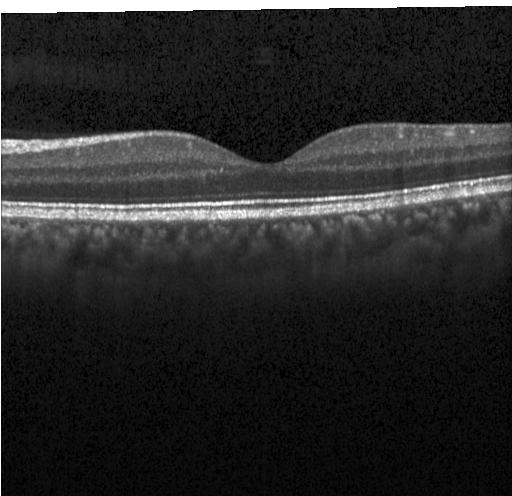

The scan shows no evidence of choroidal neovascularization, diabetic macular edema, or drusen.